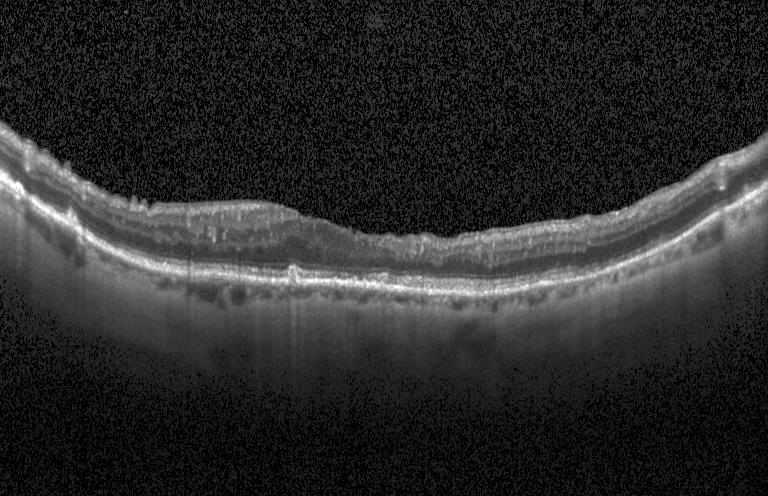

Dx: drusen.